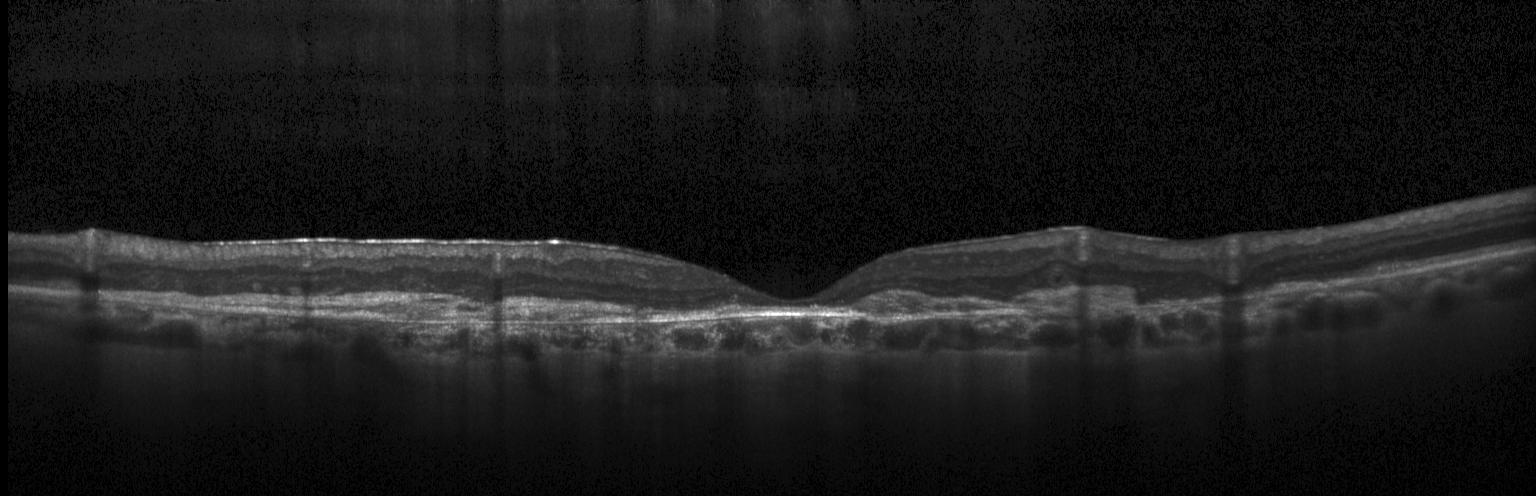
OCT B-scan showing a choroidal neovascular membrane.